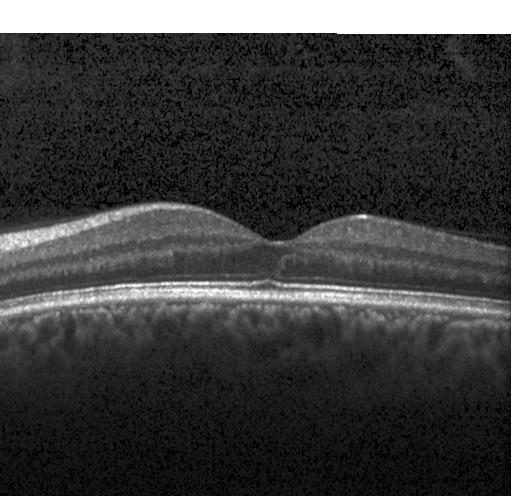 OCT B-scan showing neither CNV, DME, nor drusen.